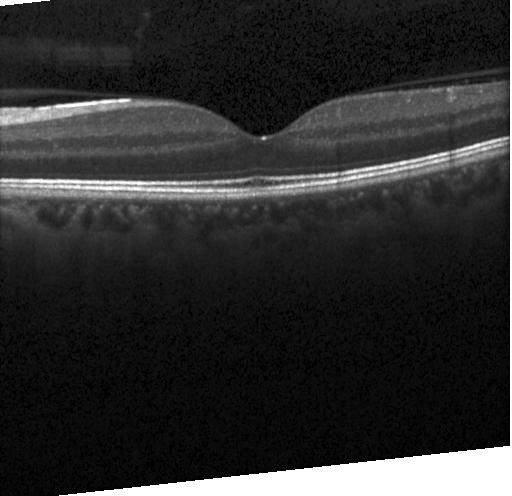

OCT finding: no choroidal neovascularization, diabetic macular edema, or drusen.